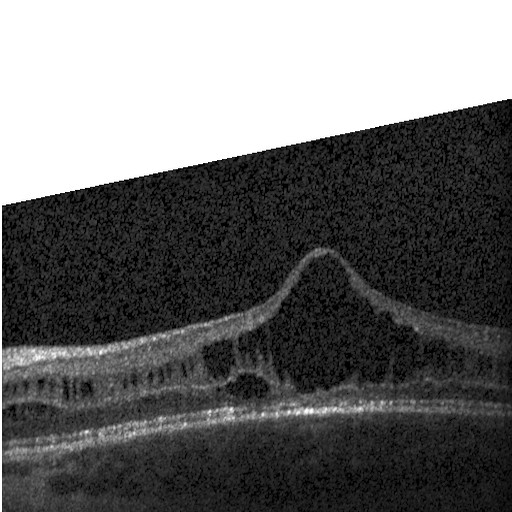
Retinal OCT B-scan.
Finding: diabetic macular edema.